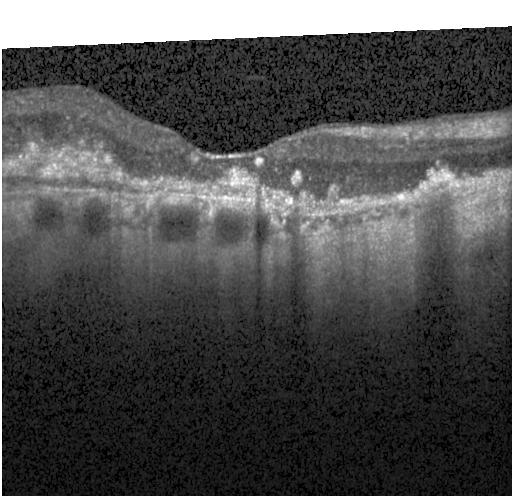 OCT B-scan; spectral-domain OCT
The scan shows a choroidal neovascular membrane.